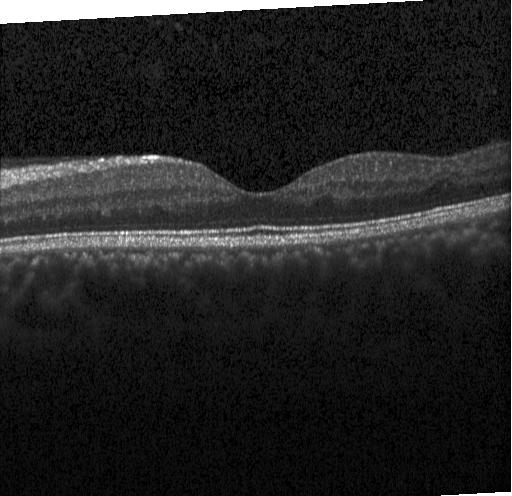
Retinal OCT cross-section
Diagnosis: no CNV, no DME, and no drusen.